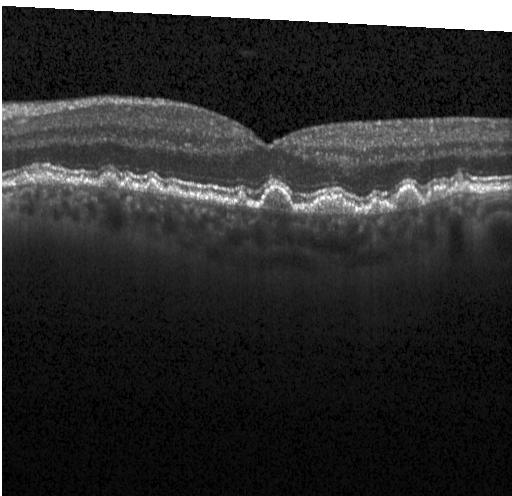 Heidelberg Spectralis OCT system. Optical coherence tomography scan. This B-scan demonstrates multiple drusen.